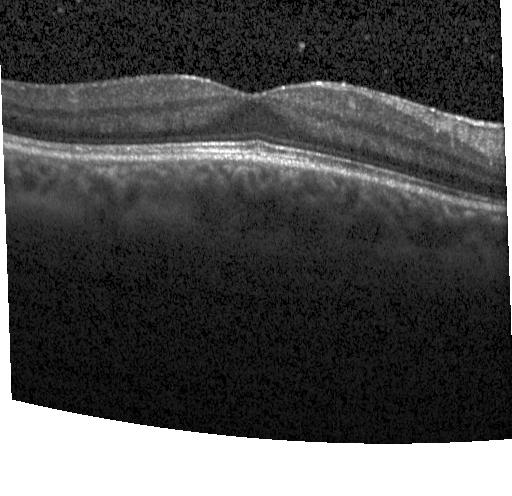
SD-OCT. Heidelberg Spectralis. Horizontal scan through the fovea. Retinal OCT cross-section — Diagnosis: neither CNV, DME, nor drusen.